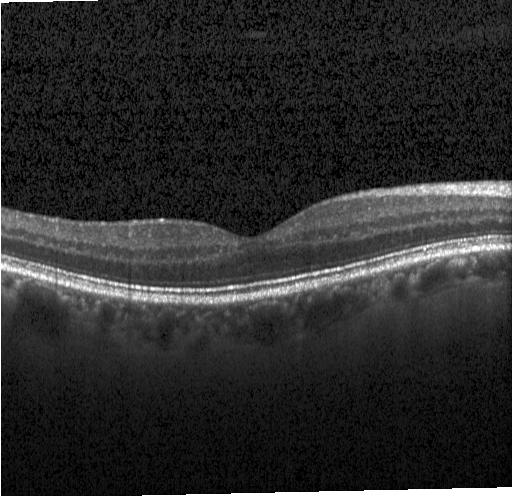

Spectral-domain OCT. Retinal OCT B-scan.
Impression: no CNV, no DME, and no drusen.